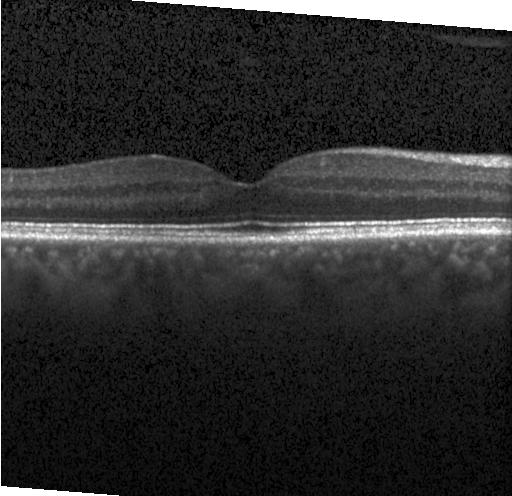
OCT finding: no CNV, DME, or drusen.